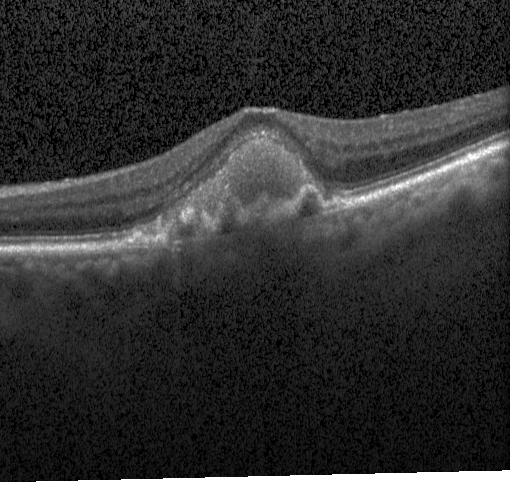 Assessment: a choroidal neovascular membrane.